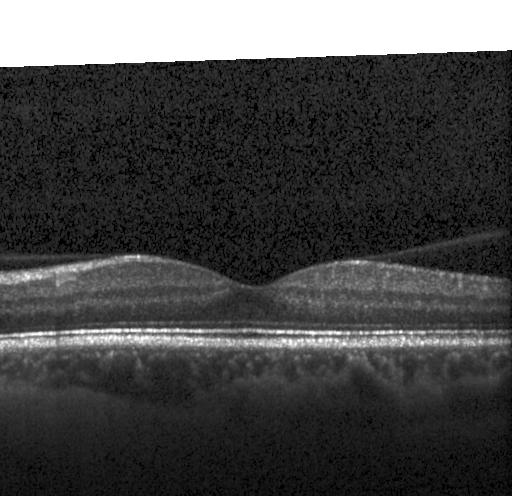
Macular OCT demonstrating no choroidal neovascularization, diabetic macular edema, or drusen.